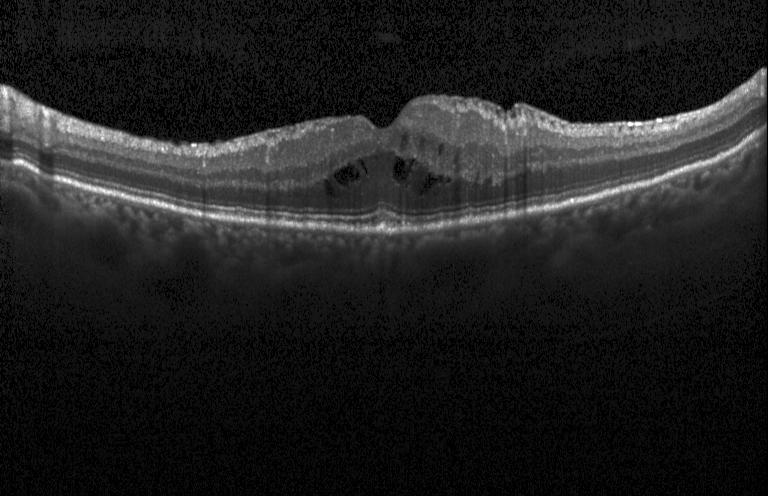
Finding: DME.